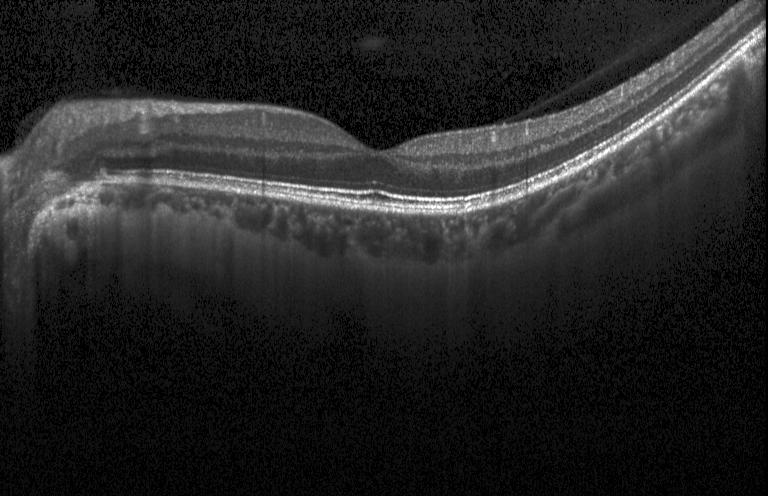

OCT scan showing no CNV, no DME, and no drusen.